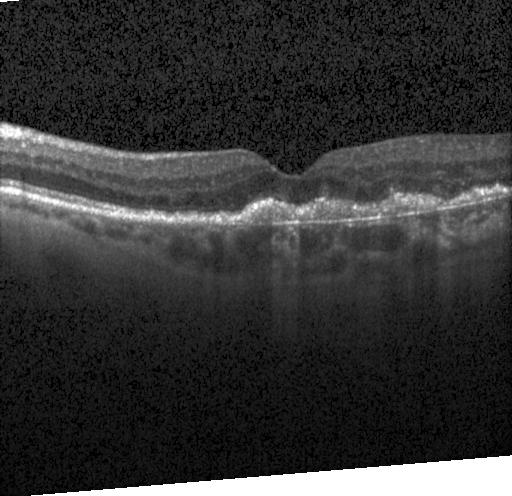 OCT scan showing choroidal neovascularization (CNV).